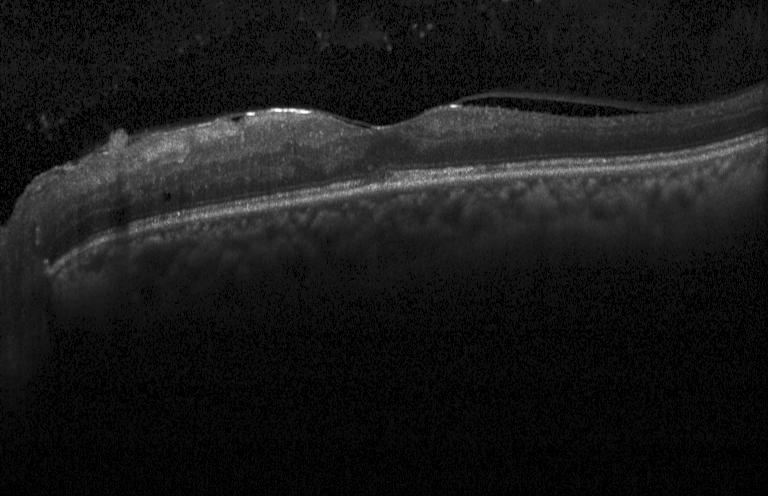
Macular scan. Spectral-domain OCT. Retinal OCT B-scan. Acquired on a Heidelberg Spectralis.
Impression: diabetic macular edema.